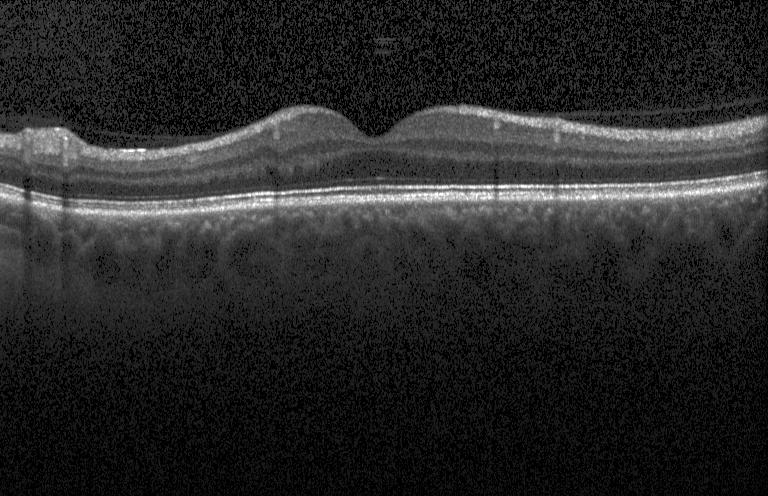
Assessment: no CNV, DME, or drusen.